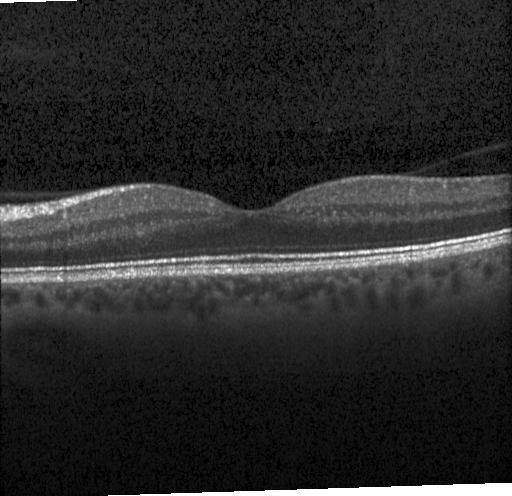

Acquired on a Heidelberg Spectralis · optical coherence tomography B-scan
Impression: no choroidal neovascularization, no diabetic macular edema, and no drusen.